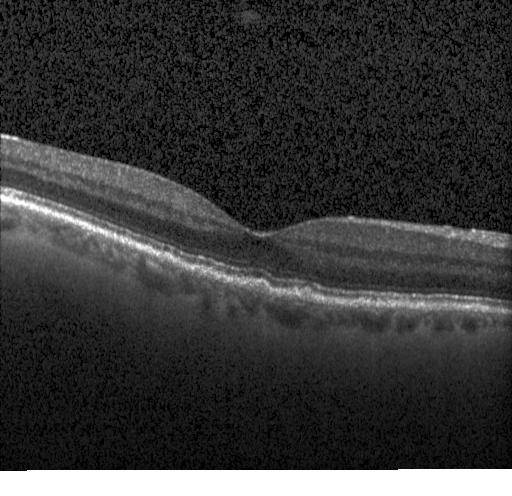

Finding: drusen.